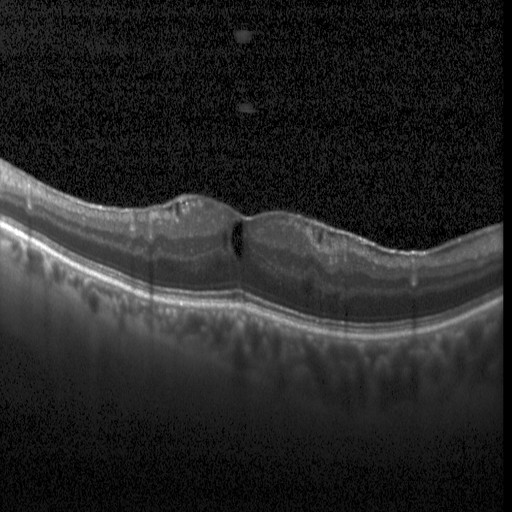
OCT B-scan showing diabetic macular edema.